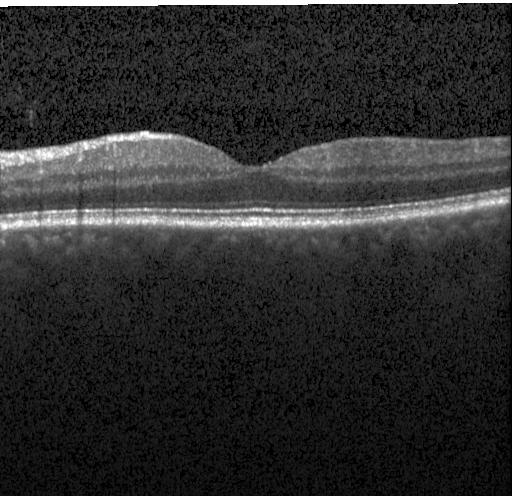

Horizontal scan through the fovea; OCT B-scan — Assessment: no CNV, DME, or drusen.